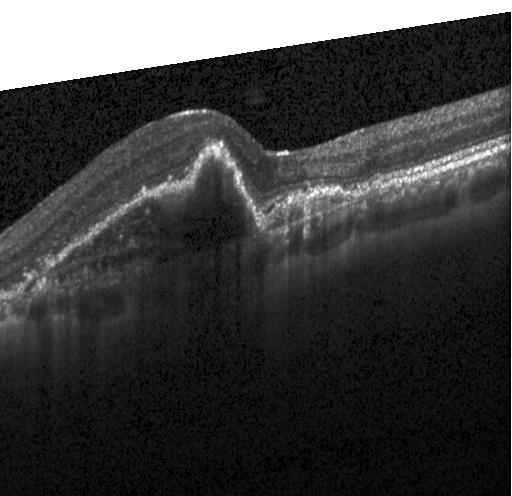 Diagnosis: choroidal neovascularization (CNV).